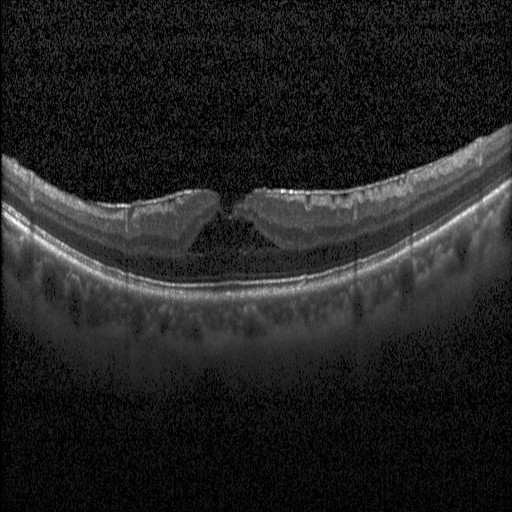
OCT line scan
Macular OCT: DME.